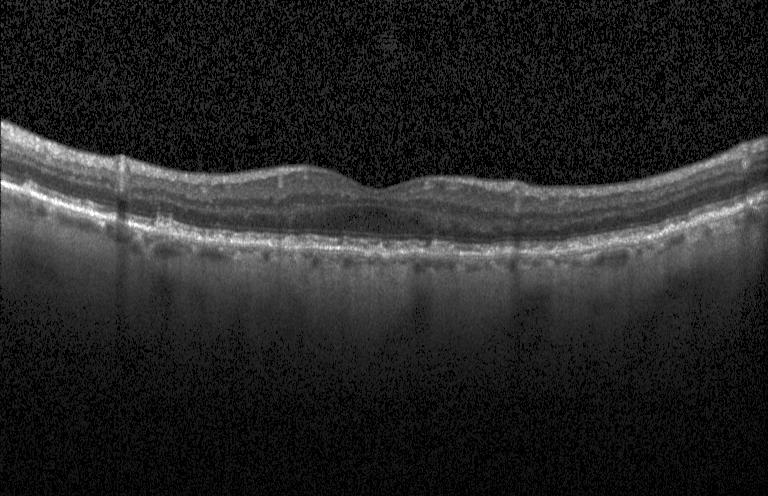
Retinal OCT cross-section showing drusen.